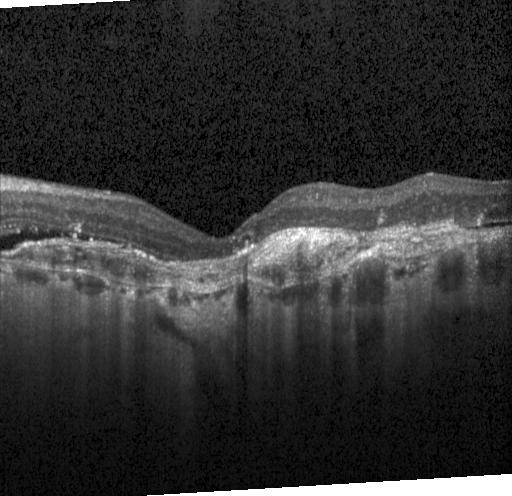 This B-scan demonstrates a choroidal neovascular membrane.